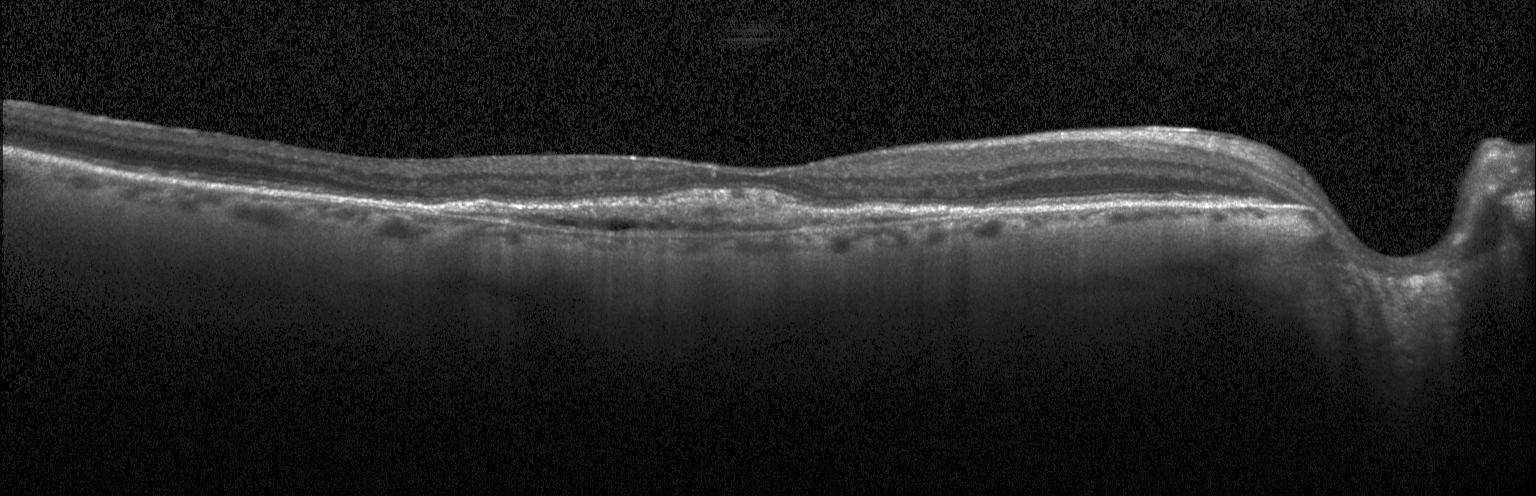 Finding: choroidal neovascularization.